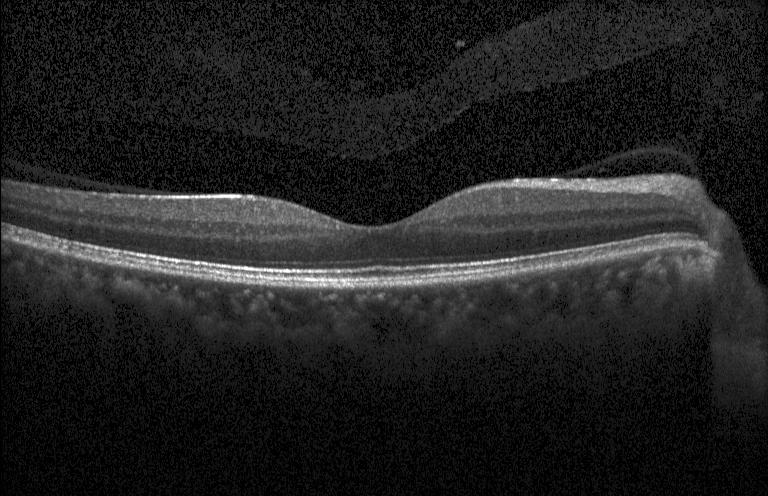

Spectral-domain optical coherence tomography · instrument: Heidelberg Spectralis · through the macula · retinal OCT cross-section
OCT finding: no choroidal neovascularization, no diabetic macular edema, and no drusen.